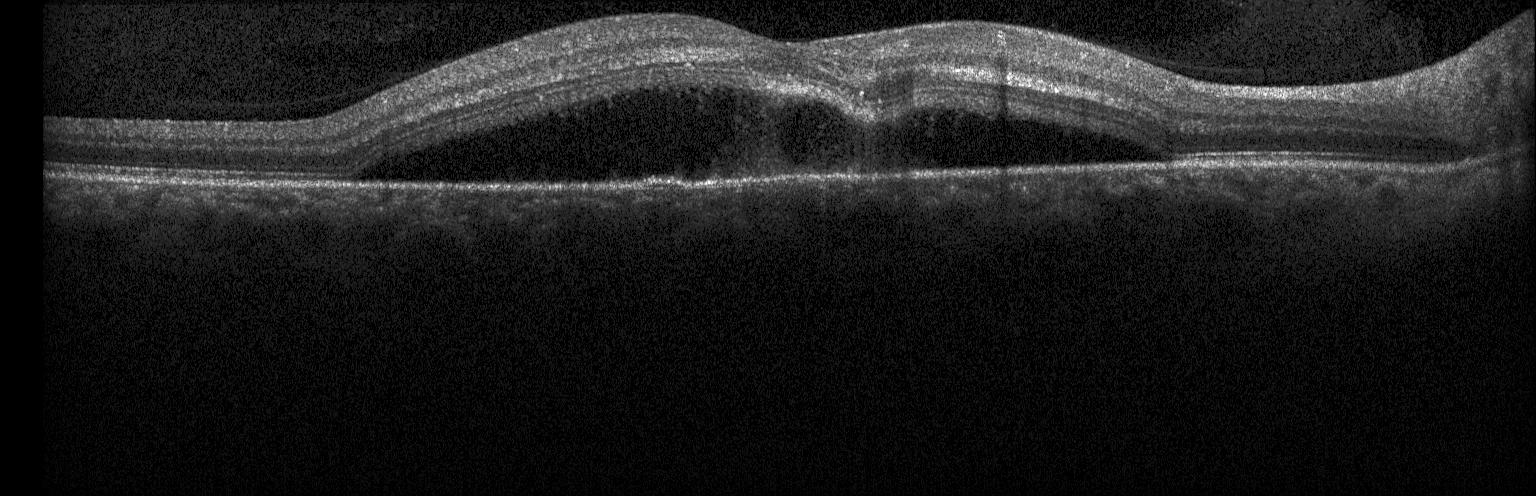 OCT B-scan showing a choroidal neovascular membrane.